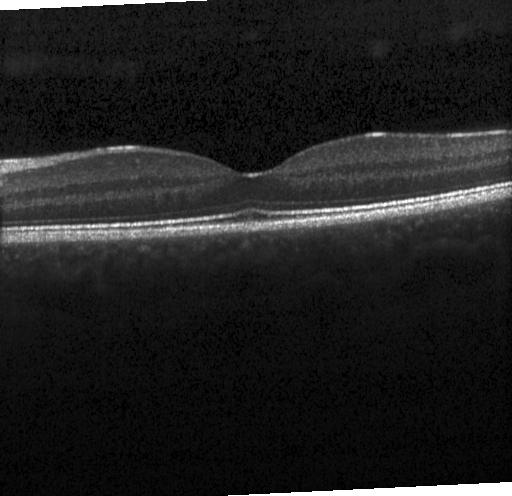

No evidence of choroidal neovascularization, diabetic macular edema, or drusen.